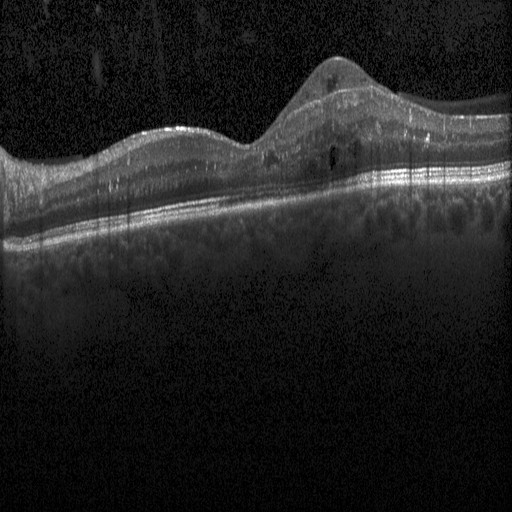
The scan shows diabetic macular edema.